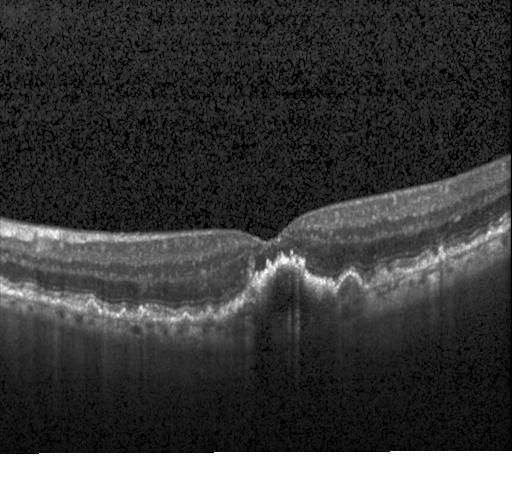

Diagnosis: CNV.